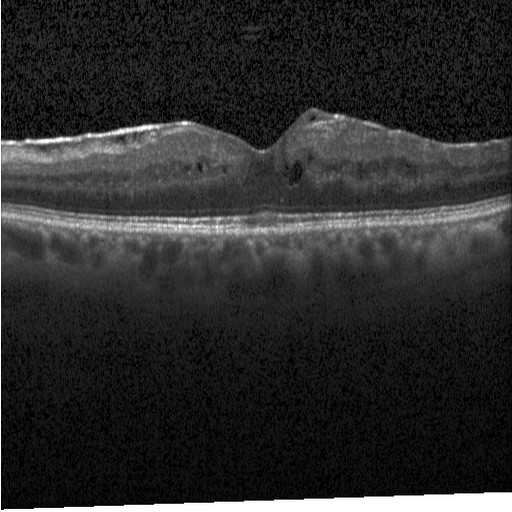
Macular OCT demonstrating diabetic macular edema (DME).